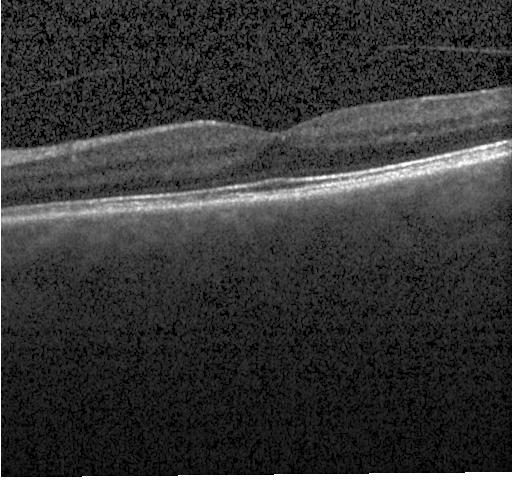

Horizontal scan through the fovea. Optical coherence tomography scan.
The scan shows no evidence of choroidal neovascularization, diabetic macular edema, or drusen.